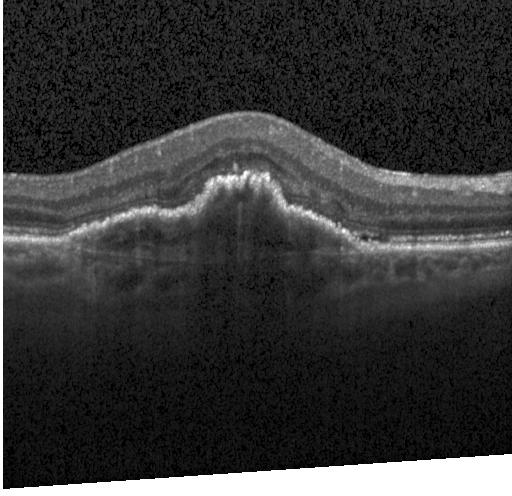
Impression: choroidal neovascularization.